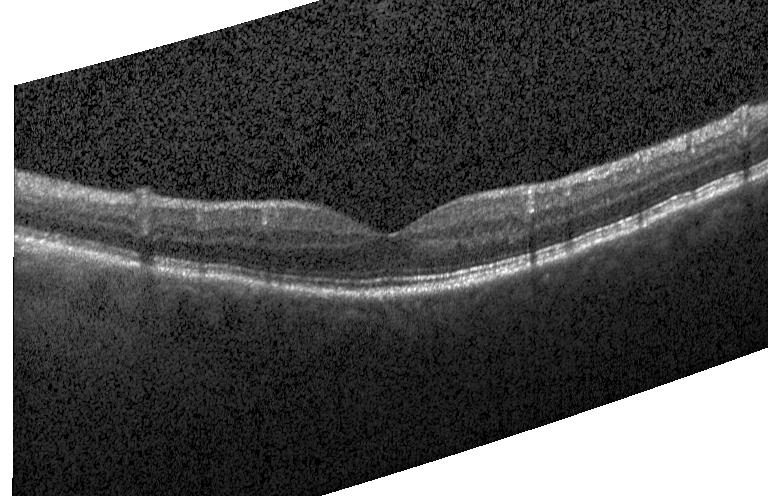 OCT B-scan · fovea-centered · spectral-domain optical coherence tomography. Diagnosis: no evidence of choroidal neovascularization, diabetic macular edema, or drusen.